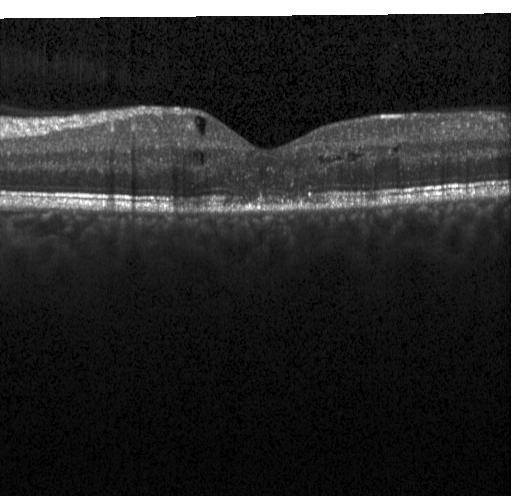 Through the macula; retinal OCT cross-section
Diagnosis: diabetic macular edema (DME).